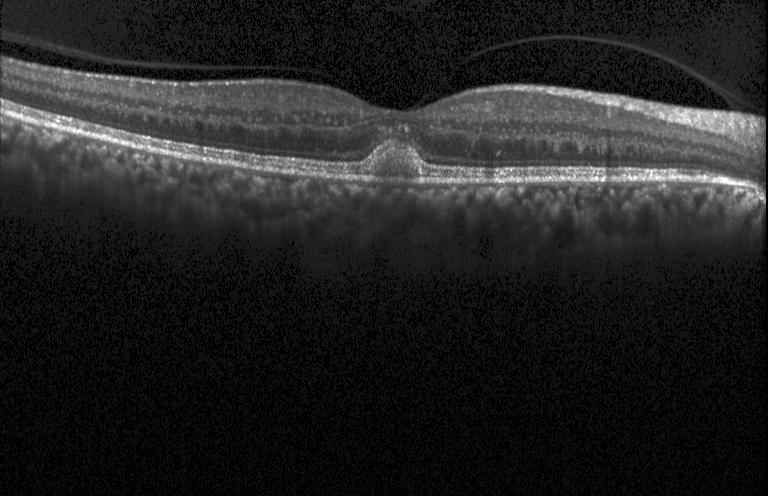
OCT B-scan showing a choroidal neovascular membrane.